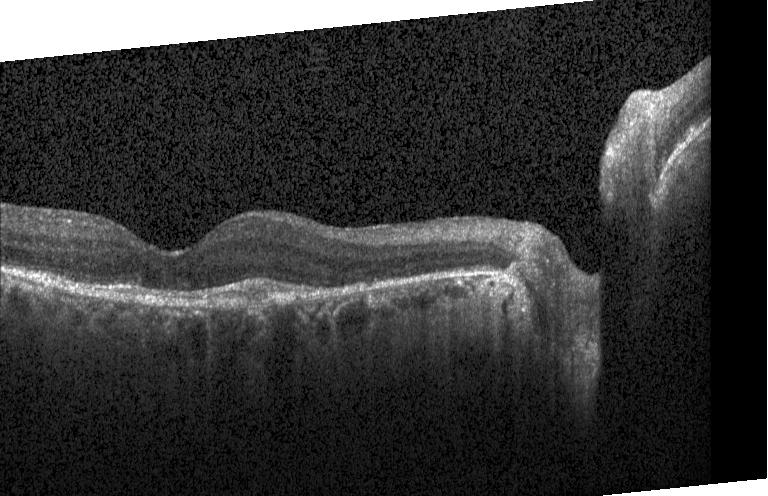 OCT B-scan — Finding: a choroidal neovascular membrane.